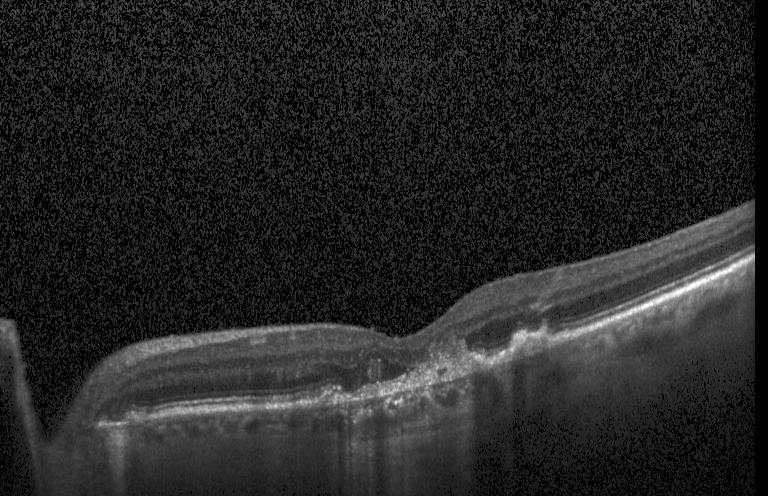 OCT scan showing a choroidal neovascular membrane.